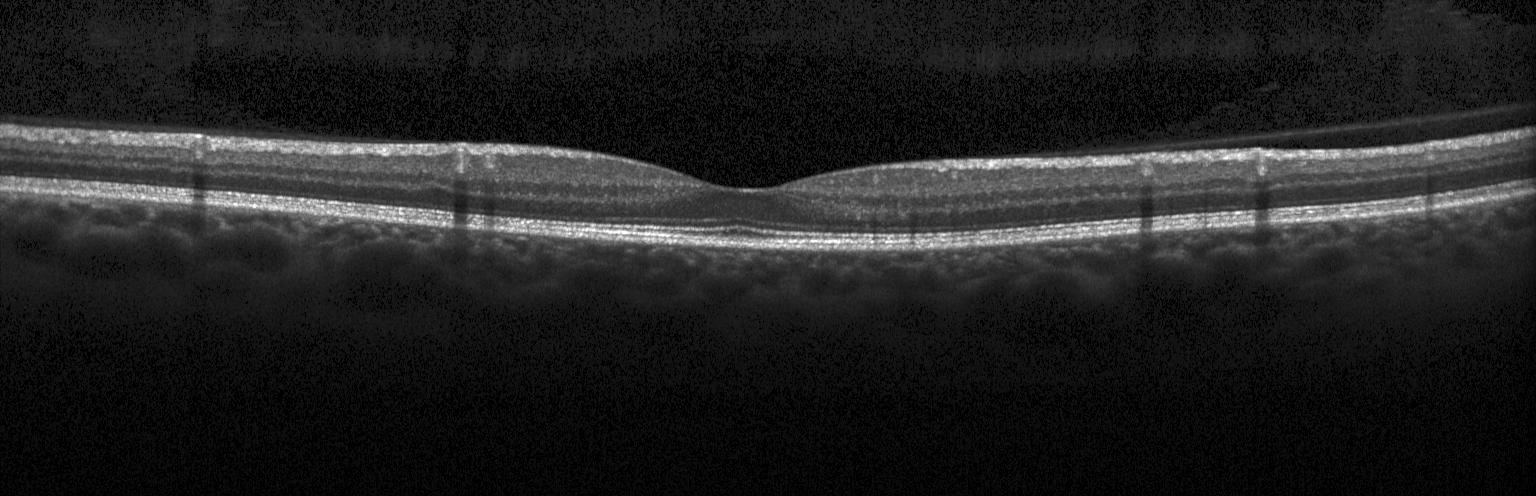
Assessment: neither choroidal neovascularization, diabetic macular edema, nor drusen.